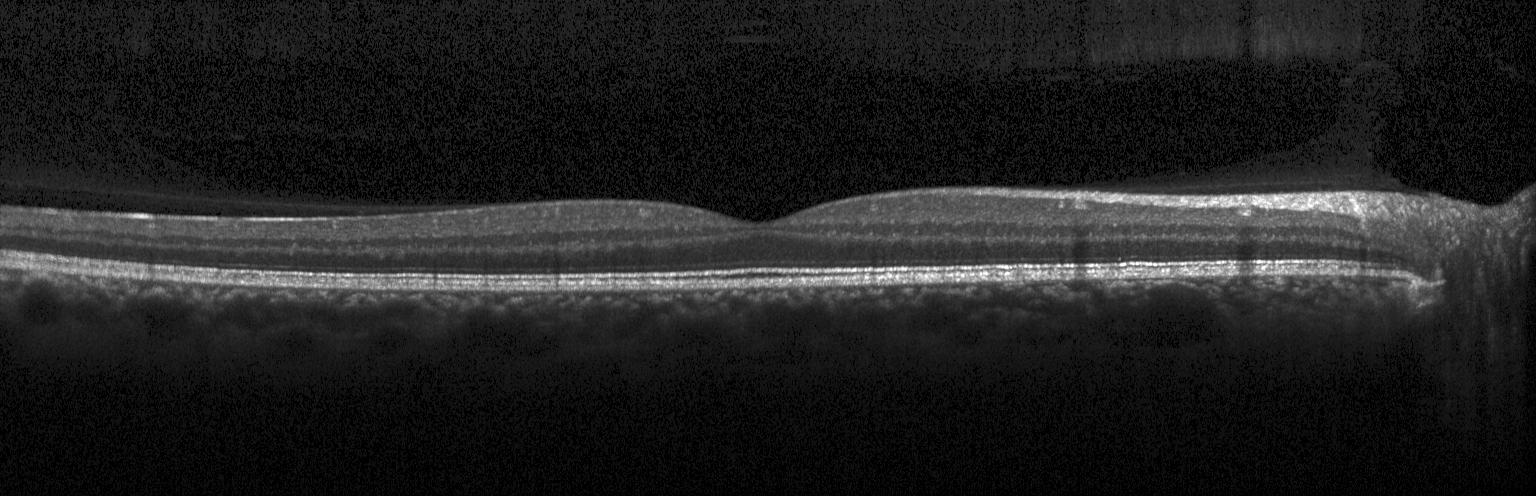

Assessment: neither choroidal neovascularization, diabetic macular edema, nor drusen.